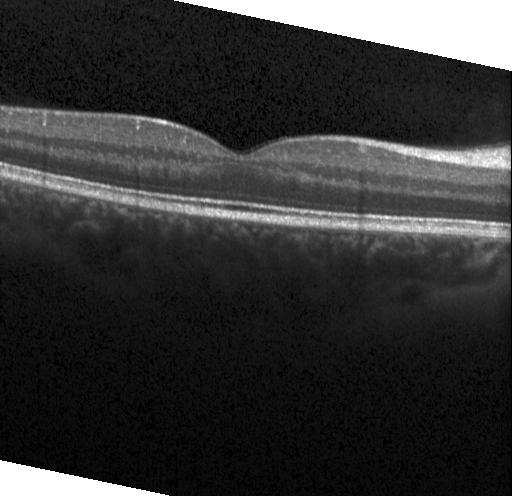

Impression: no CNV, no DME, and no drusen.